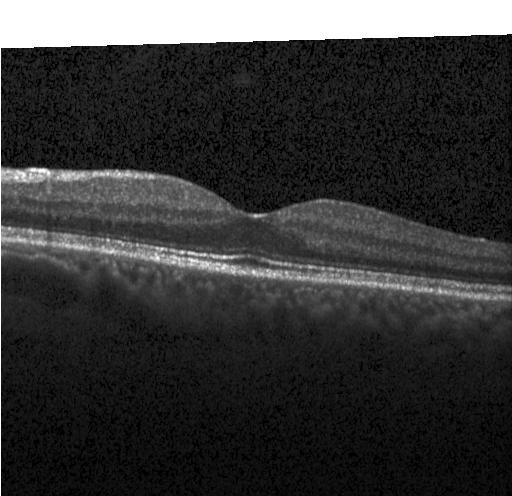
Impression: no evidence of CNV, DME, or drusen.